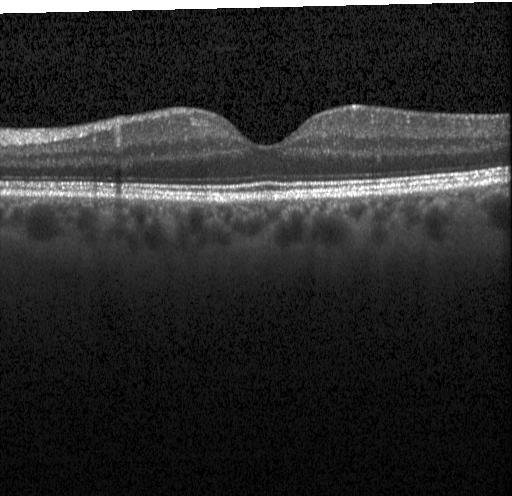 Optical coherence tomography scan. Heidelberg Spectralis.
Diagnosis: neither choroidal neovascularization, diabetic macular edema, nor drusen.